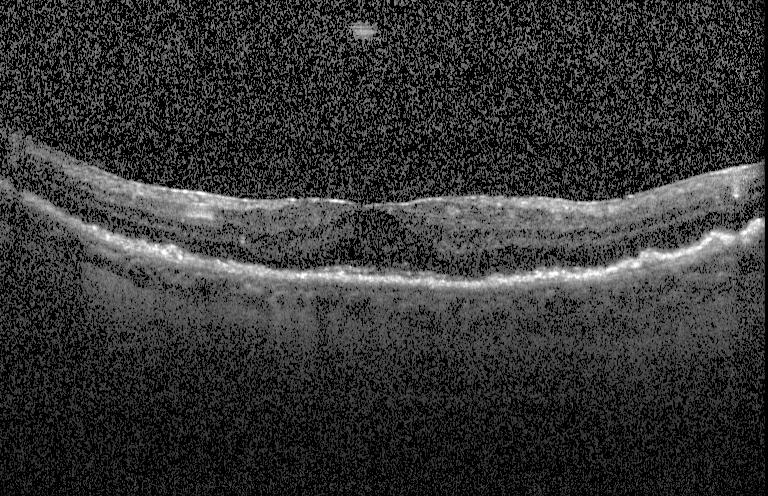

SD-OCT. Acquired on a Heidelberg Spectralis. OCT B-scan.
Finding: choroidal neovascularization.